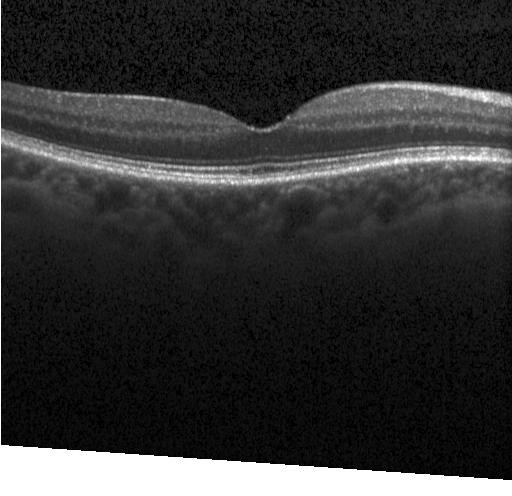

Centered on the fovea; retinal OCT cross-section — Impression: no evidence of CNV, DME, or drusen.